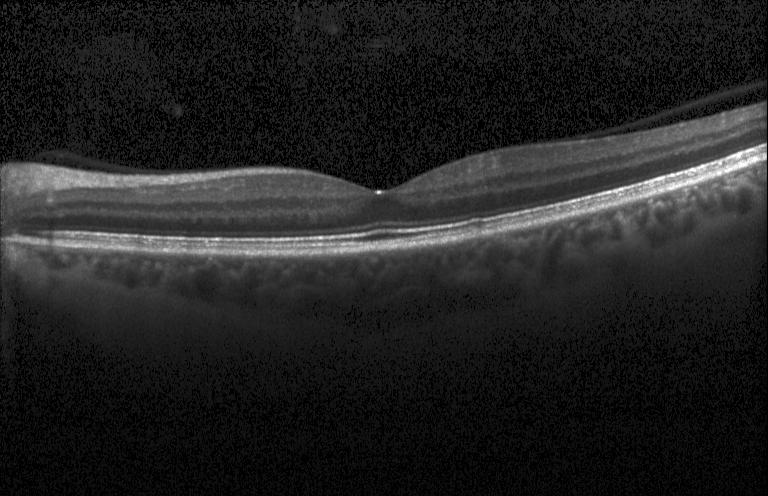
OCT B-scan.
OCT finding: no choroidal neovascularization, diabetic macular edema, or drusen.